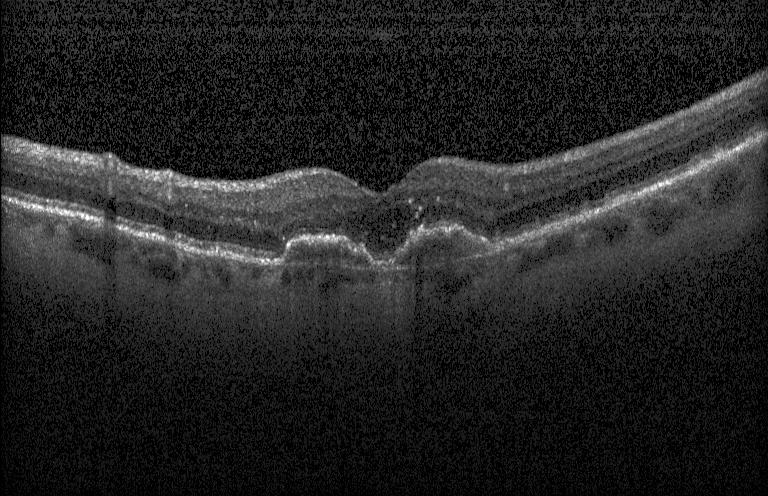
Optical coherence tomography scan.
Finding: a choroidal neovascular membrane.